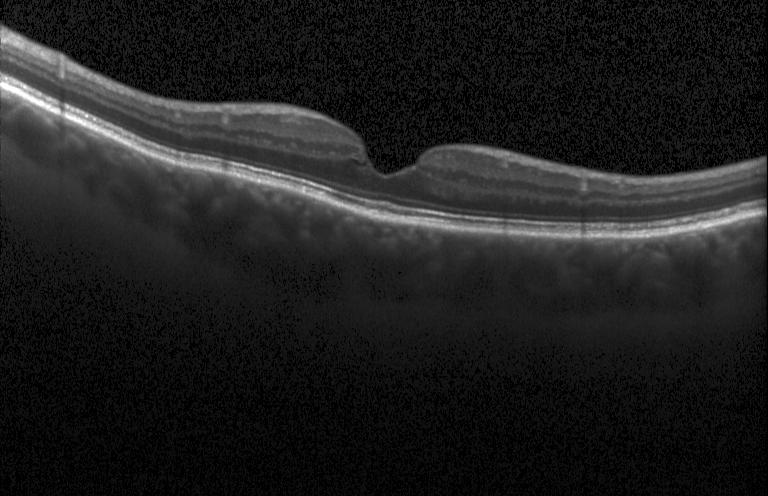
OCT line scan; instrument: Heidelberg Spectralis. This B-scan demonstrates diabetic macular edema (DME).